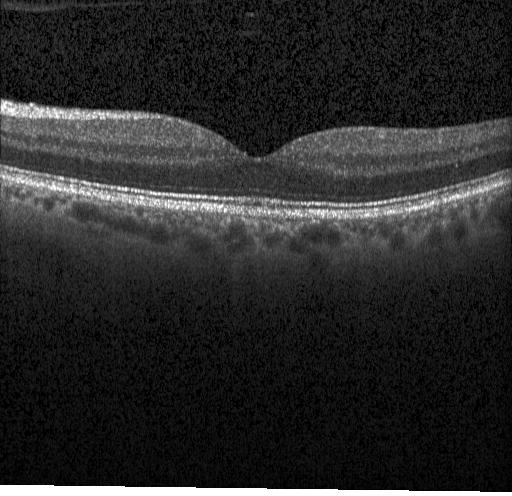

Optical coherence tomography scan — Diagnosis: no CNV, no DME, and no drusen.